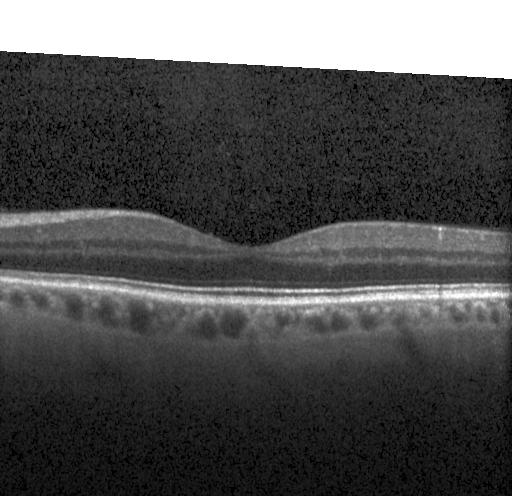
Macular OCT: neither CNV, DME, nor drusen.